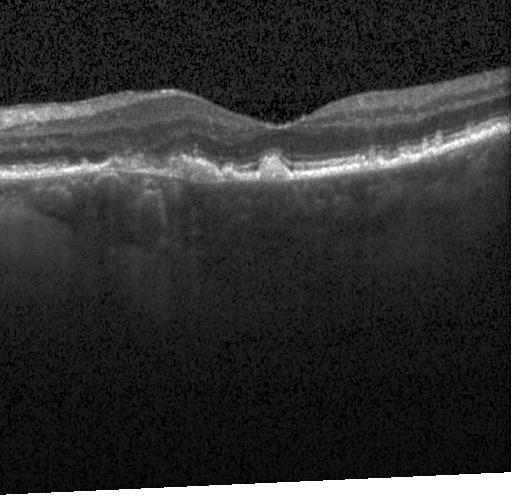

Impression: a choroidal neovascular membrane.